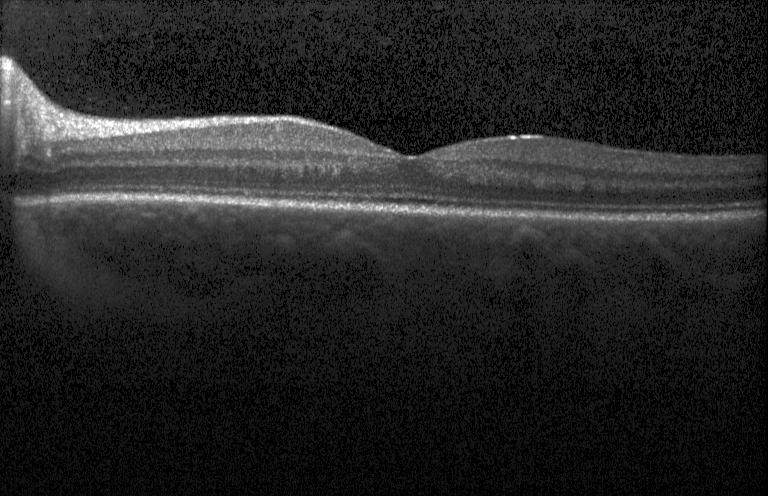 SD-OCT, optical coherence tomography scan — Diagnosis: no evidence of choroidal neovascularization, diabetic macular edema, or drusen.